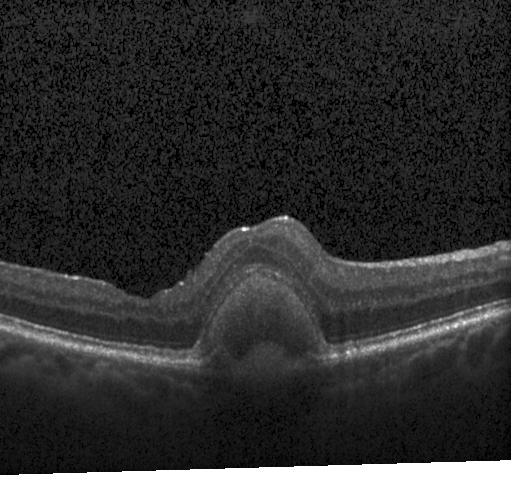
Optical coherence tomography B-scan.
Diagnosis: choroidal neovascularization.